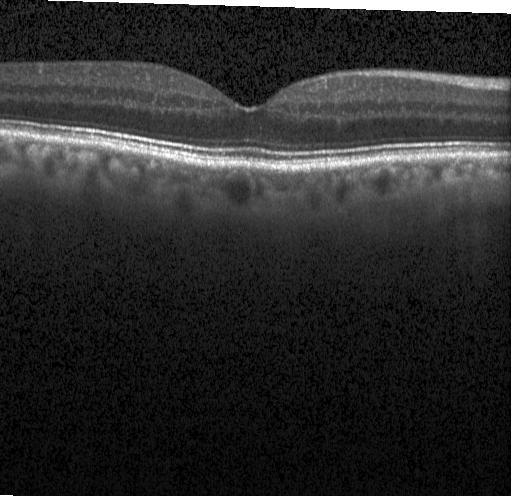

Impression: neither CNV, DME, nor drusen.